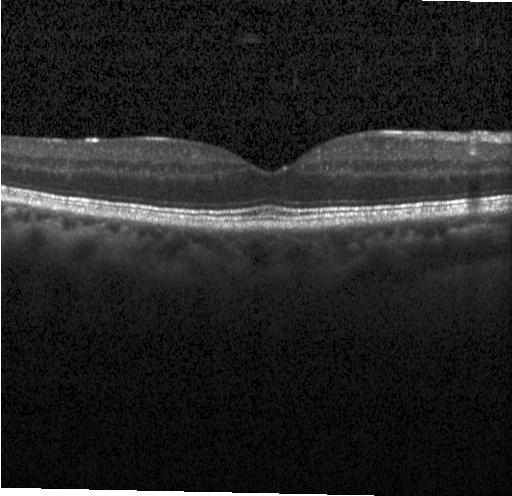 Spectral-domain OCT. Heidelberg Spectralis. OCT line scan
This B-scan demonstrates no CNV, DME, or drusen.